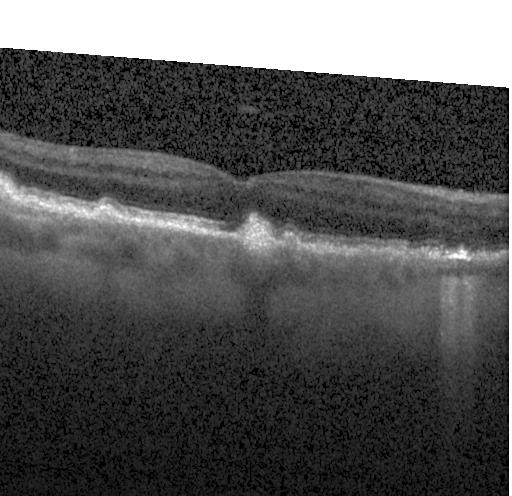

SD-OCT. Heidelberg Spectralis. Optical coherence tomography scan. Horizontal scan through the fovea. The scan shows drusen.